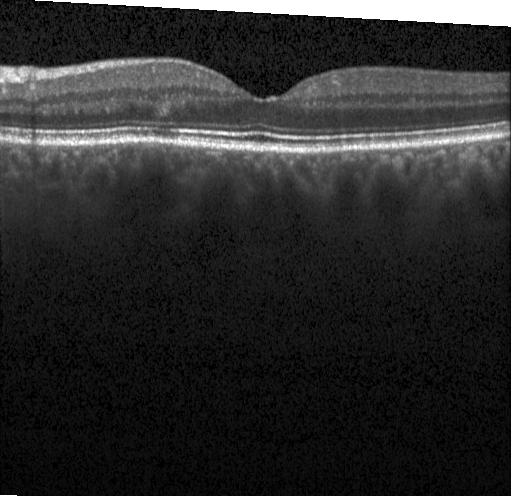 Horizontal scan through the fovea. Retinal OCT B-scan.
Impression: no choroidal neovascularization, diabetic macular edema, or drusen.